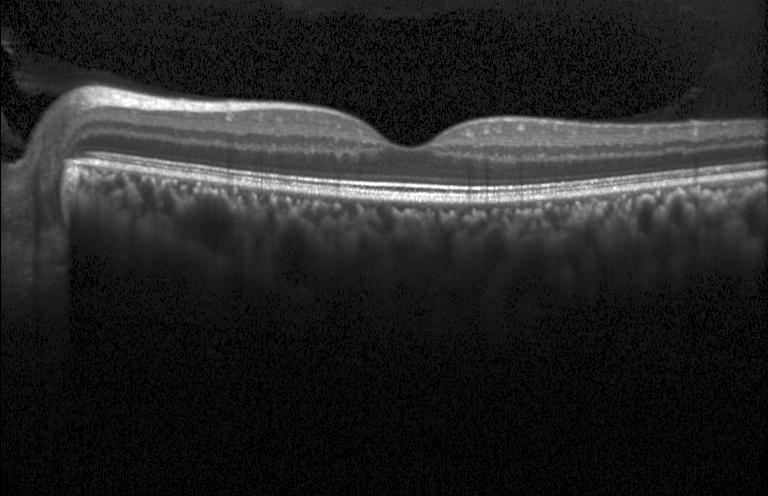 Retinal OCT cross-section; acquired on a Heidelberg Spectralis; spectral-domain OCT; centered on the fovea — Impression: no choroidal neovascularization, no diabetic macular edema, and no drusen.